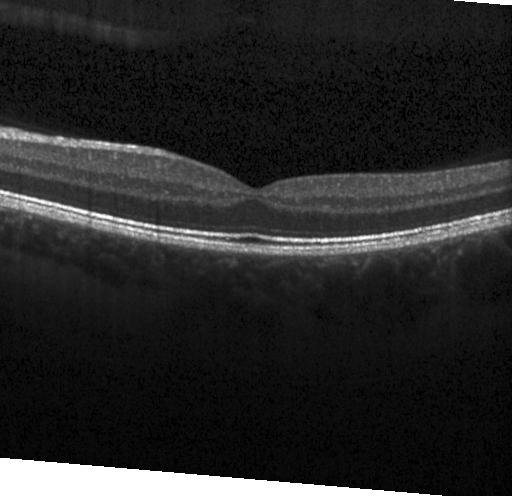
SD-OCT · optical coherence tomography B-scan · centered on the fovea
Assessment: no CNV, DME, or drusen.